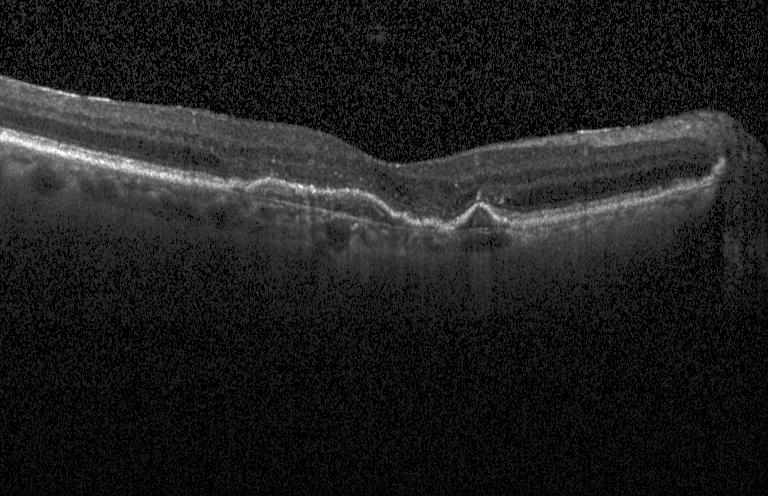

Diagnosis: a choroidal neovascular membrane.